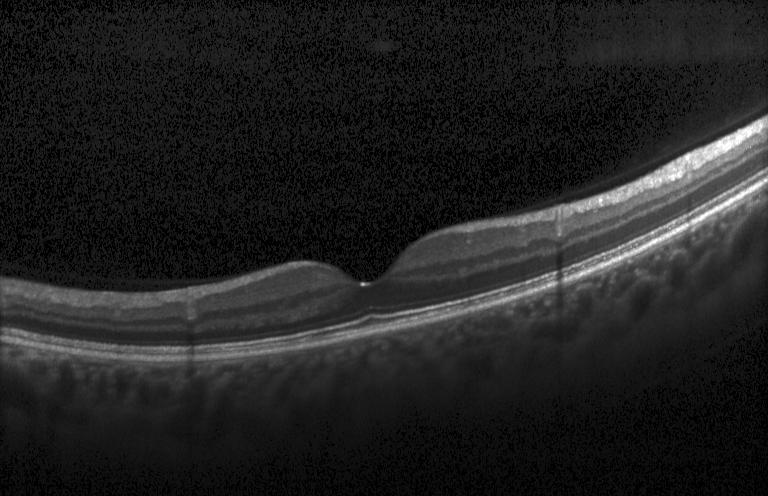 OCT line scan.
Diagnosis: no choroidal neovascularization, diabetic macular edema, or drusen.